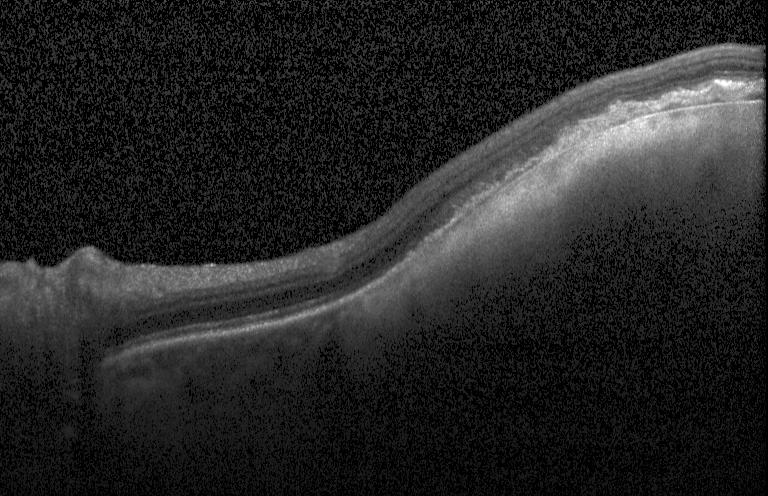
Diagnosis: choroidal neovascularization (CNV).